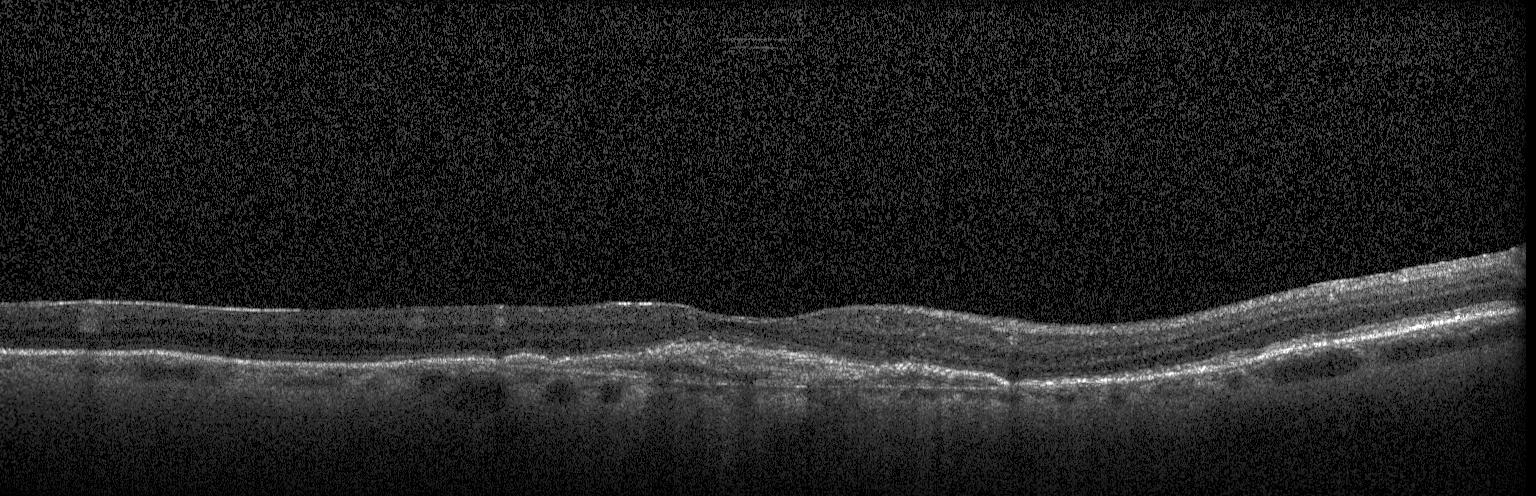
Acquired on a Heidelberg Spectralis. Macular scan. Retinal OCT cross-section
Choroidal neovascularization.